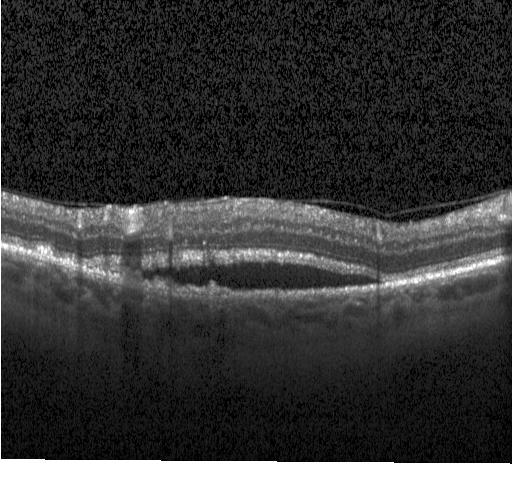

Centered on the fovea. Acquired on a Heidelberg Spectralis. Retinal OCT B-scan — Dx: a choroidal neovascular membrane.